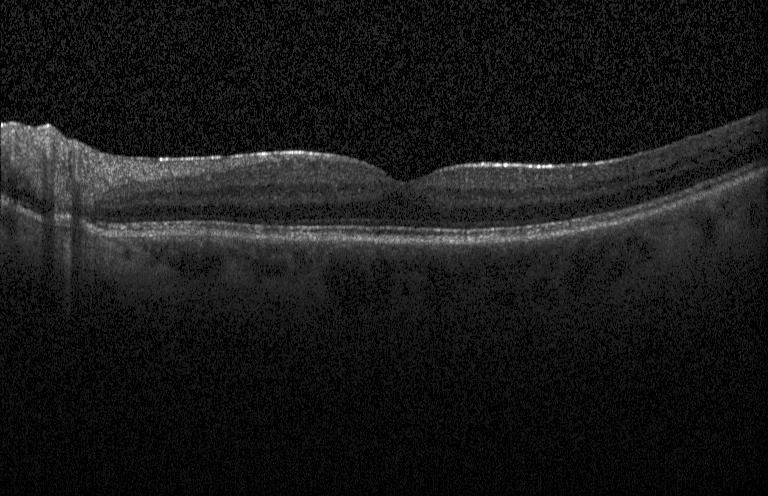 Impression: no choroidal neovascularization, no diabetic macular edema, and no drusen.